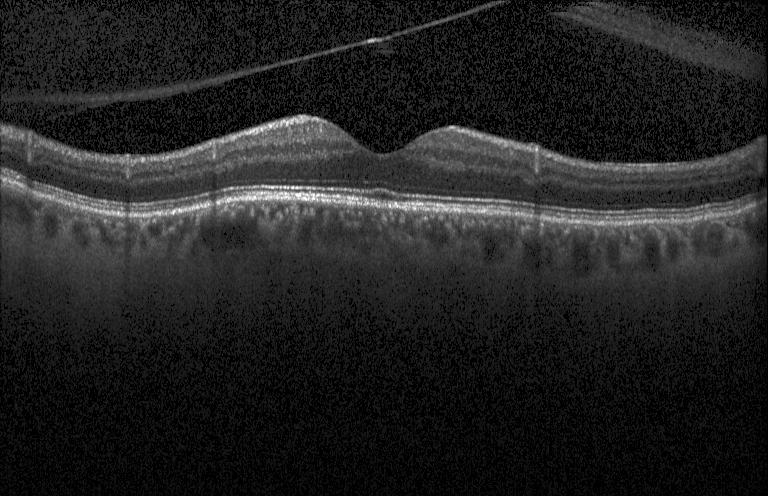

Macular OCT: neither CNV, DME, nor drusen.